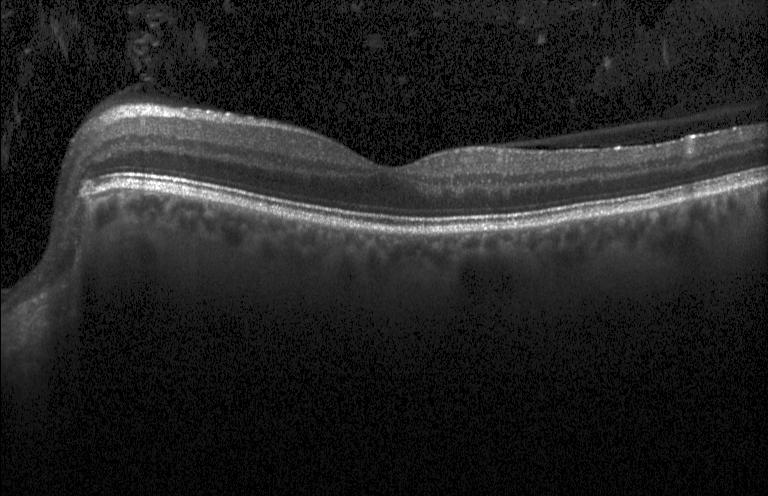
Optical coherence tomography scan.
No choroidal neovascularization, no diabetic macular edema, and no drusen.